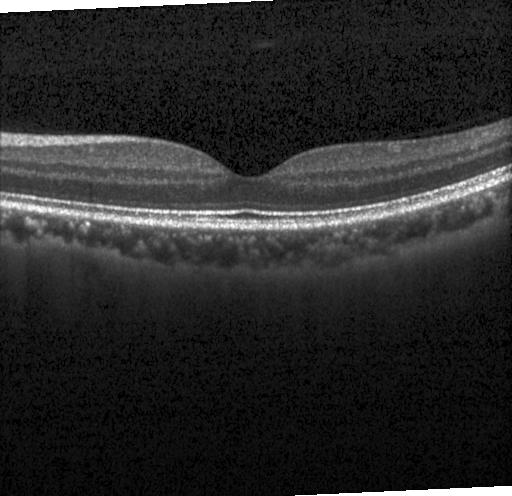

Assessment: no choroidal neovascularization, no diabetic macular edema, and no drusen.